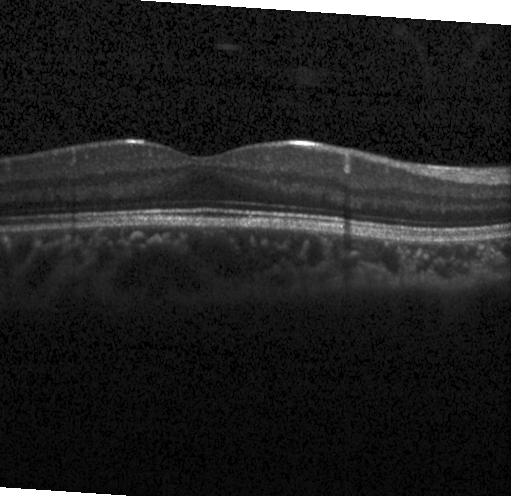
Spectral-domain optical coherence tomography · retinal OCT B-scan.
Diagnosis: no evidence of choroidal neovascularization, diabetic macular edema, or drusen.